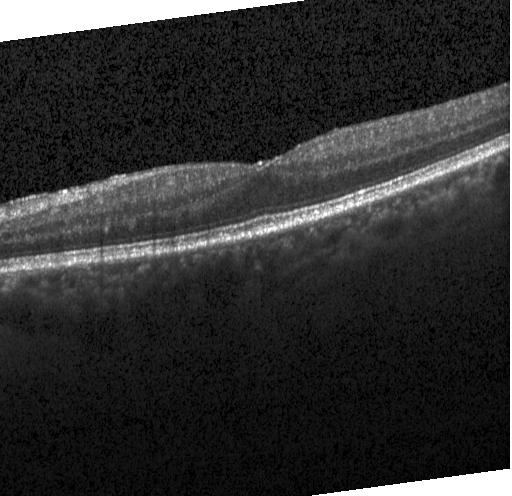

Retinal OCT cross-section · SD-OCT.
This B-scan demonstrates no choroidal neovascularization, diabetic macular edema, or drusen.